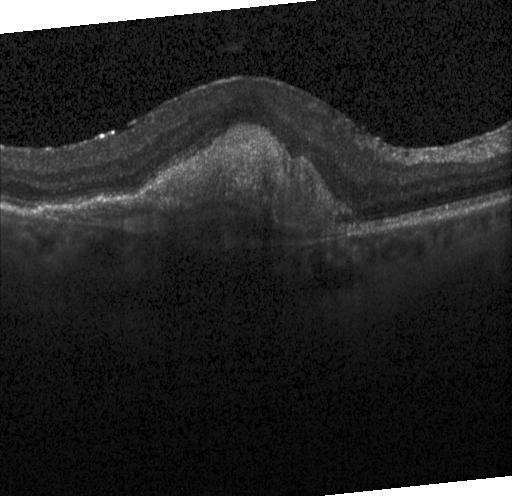 Diagnosis: choroidal neovascularization.